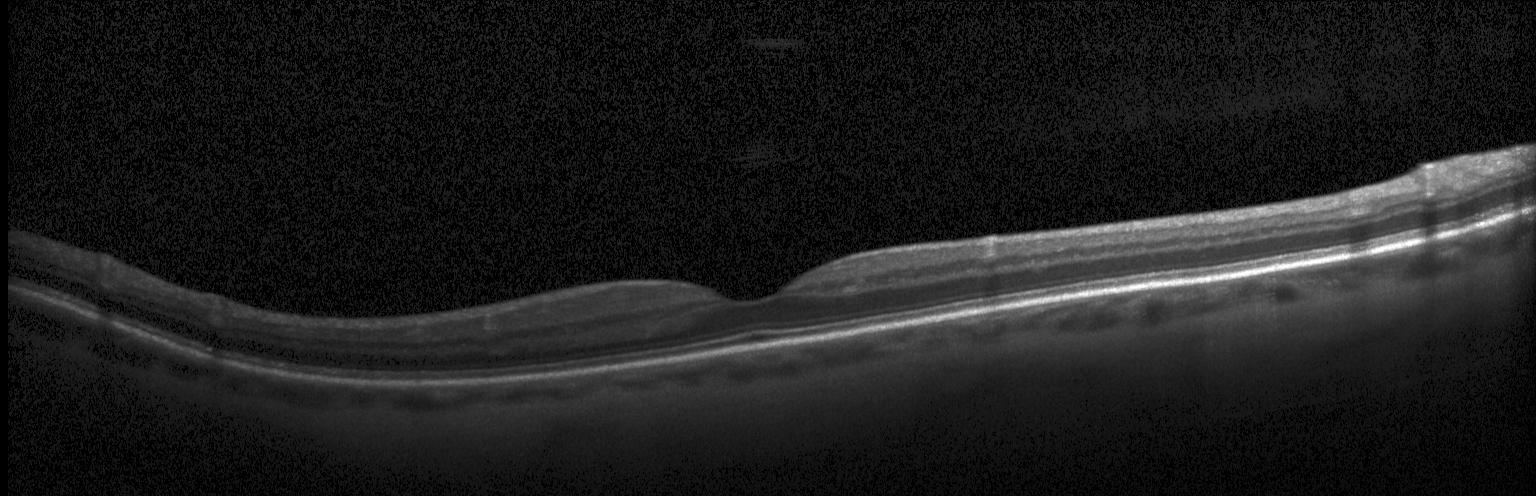
OCT finding: no evidence of CNV, DME, or drusen.